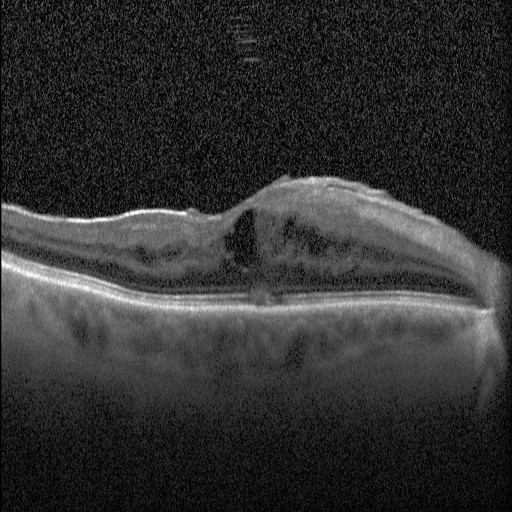
Spectral-domain OCT B-scan: diabetic macular edema.